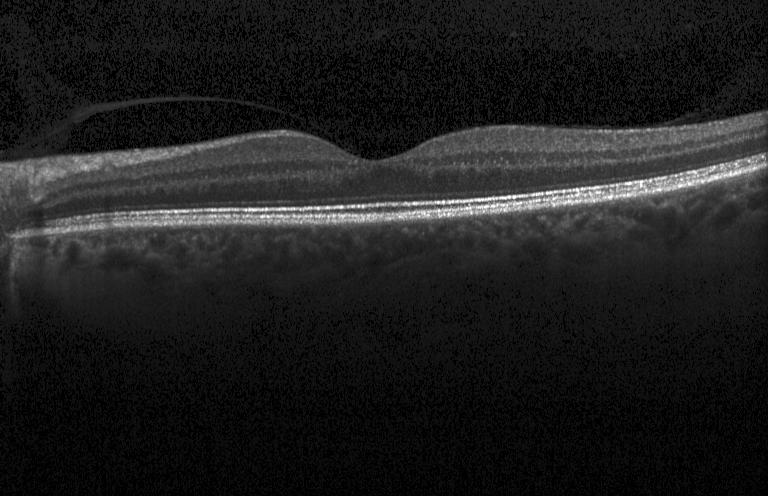
Impression: neither choroidal neovascularization, diabetic macular edema, nor drusen.